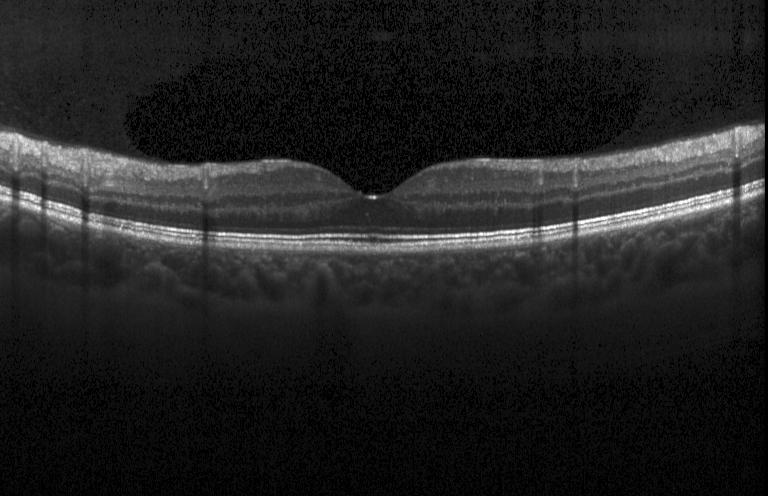 Retinal OCT B-scan; centered on the fovea. Assessment: no CNV, DME, or drusen.